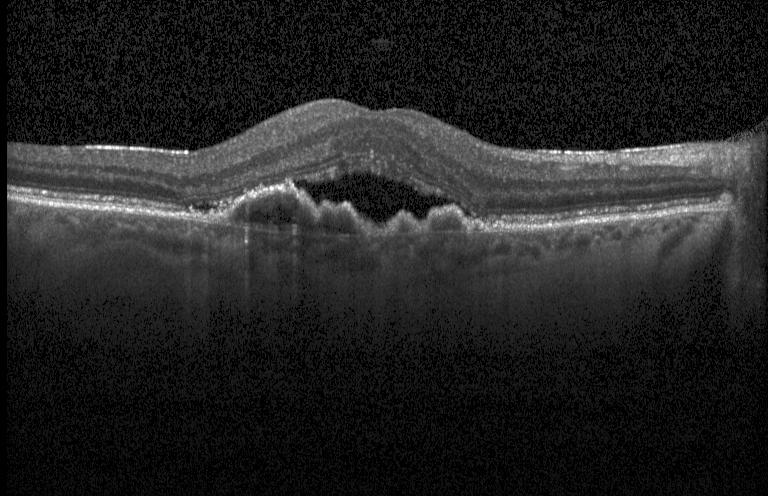
Retinal OCT B-scan. SD-OCT. Assessment: a choroidal neovascular membrane.